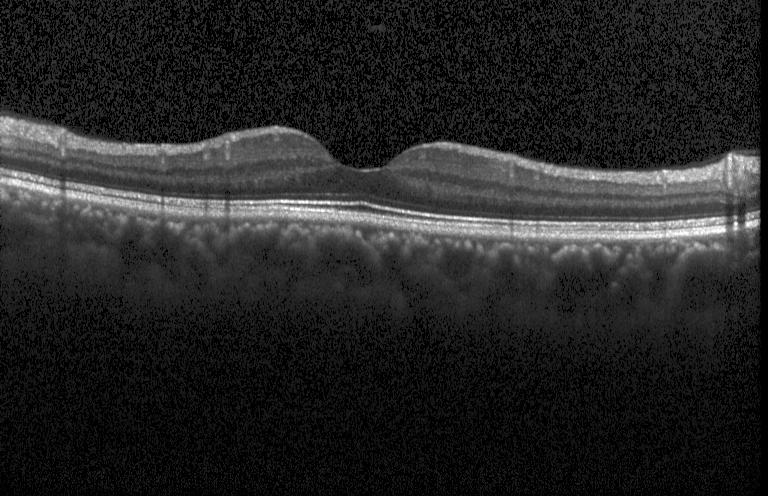

OCT B-scan. Heidelberg Spectralis. SD-OCT
No evidence of CNV, DME, or drusen.